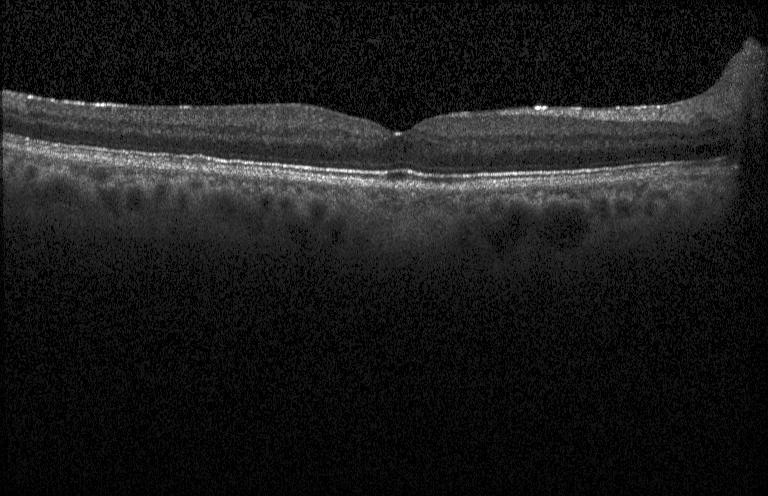 Finding: neither CNV, DME, nor drusen.